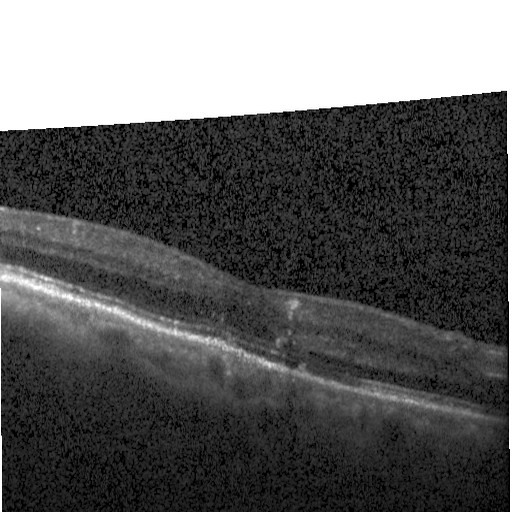
Heidelberg Spectralis OCT system; OCT B-scan; SD-OCT; horizontal scan through the fovea — Diagnosis: diabetic macular edema.